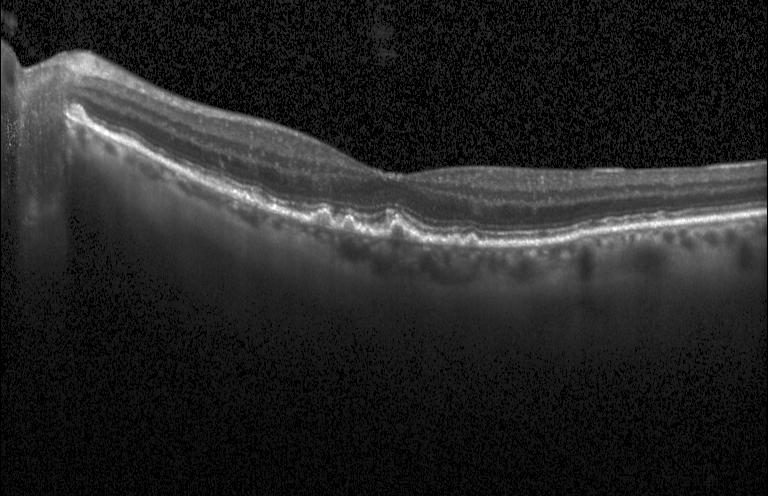

Macular scan; Heidelberg Spectralis; optical coherence tomography B-scan
This B-scan demonstrates drusen.